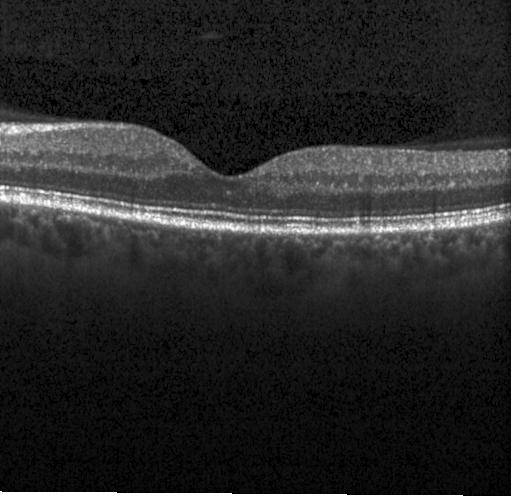

Dx: no choroidal neovascularization, diabetic macular edema, or drusen.